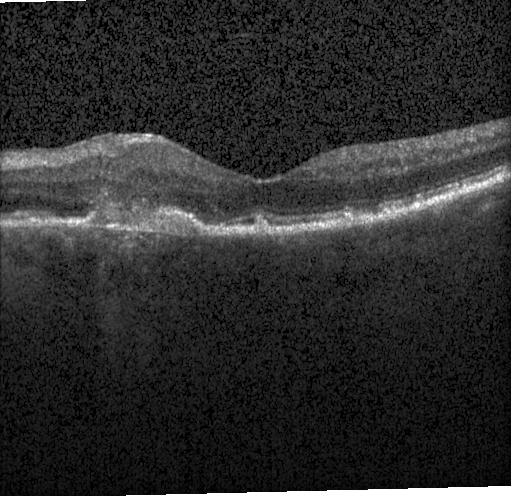

SD-OCT; OCT line scan. Finding: a choroidal neovascular membrane.